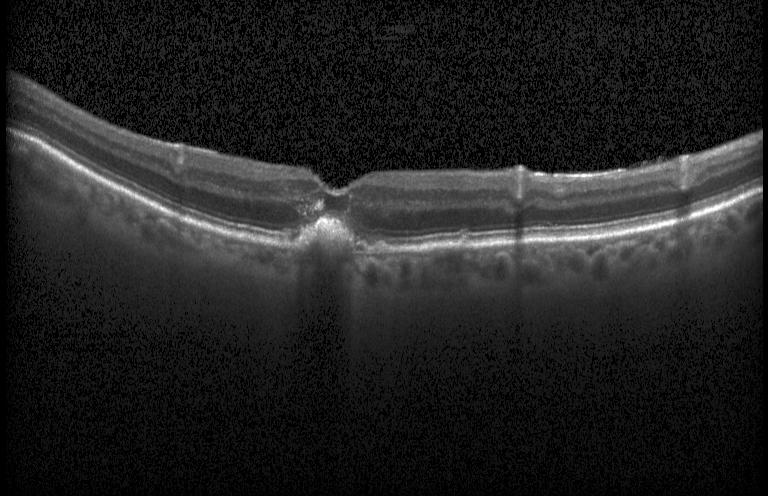 Diagnosis: a choroidal neovascular membrane.